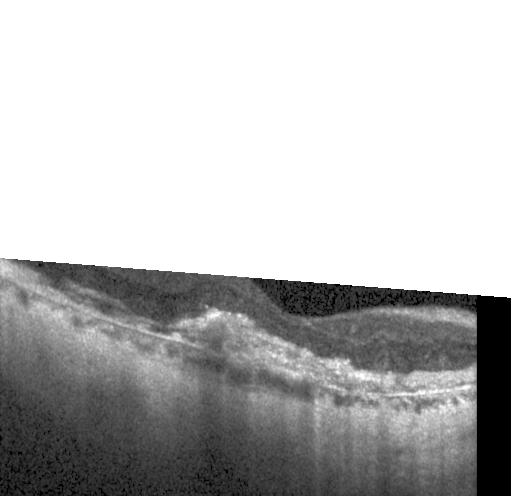

Macular scan, spectral-domain OCT, OCT line scan. Diagnosis: CNV.